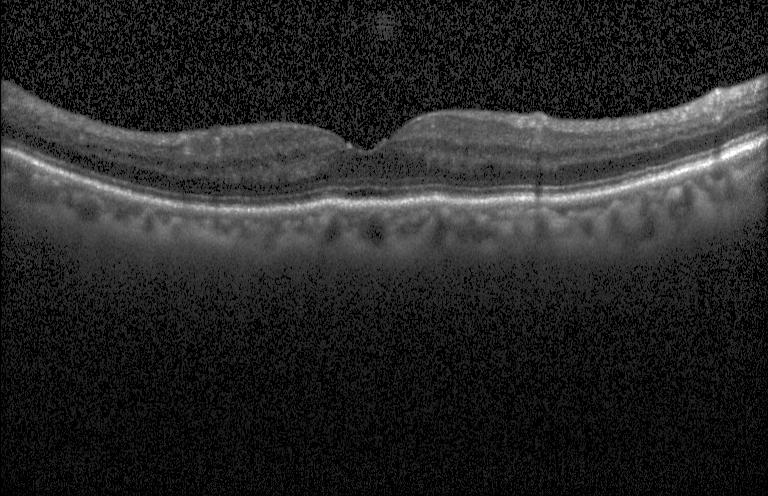

Impression: no choroidal neovascularization, diabetic macular edema, or drusen.